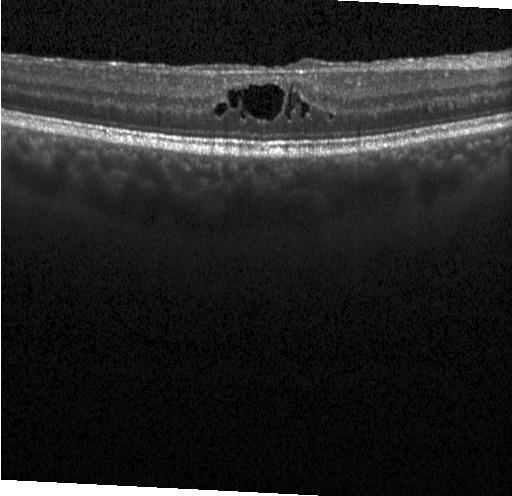 Impression: DME.